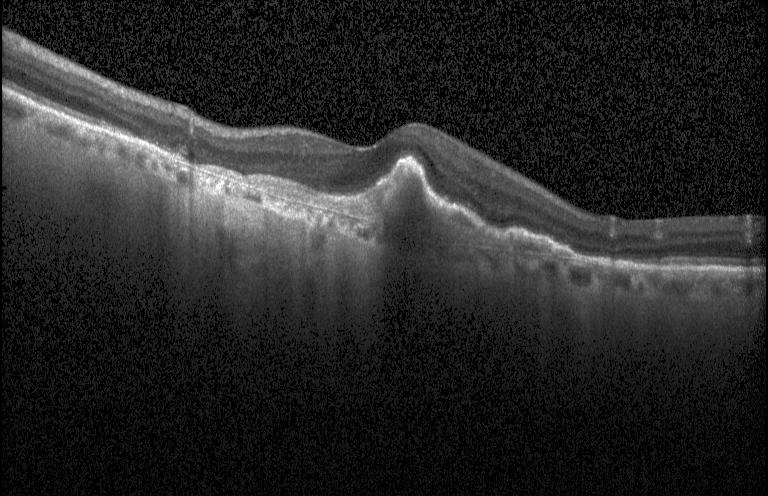

Optical coherence tomography B-scan.
Assessment: a choroidal neovascular membrane.